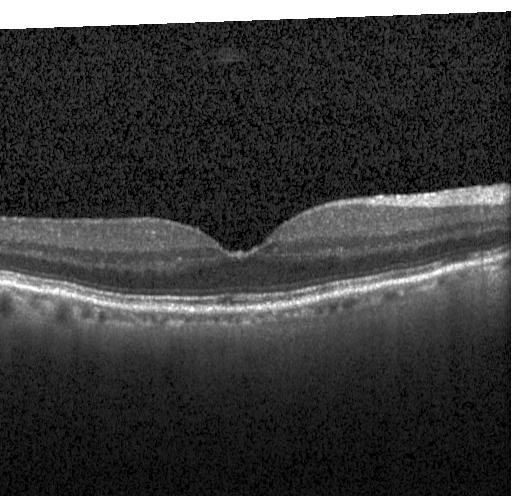
OCT B-scan. Instrument: Heidelberg Spectralis. Spectral-domain OCT. Dx: no choroidal neovascularization, no diabetic macular edema, and no drusen.